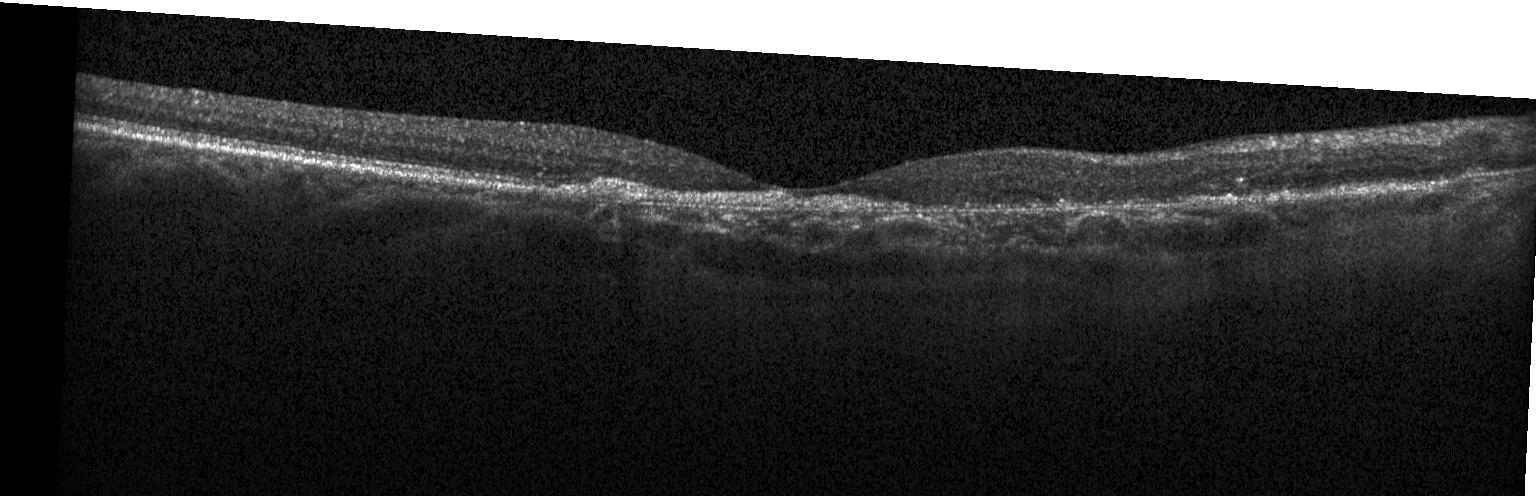

Diagnosis: CNV.